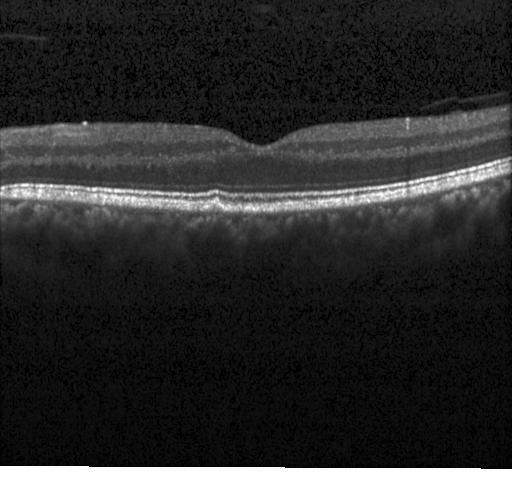 Heidelberg Spectralis OCT system. SD-OCT. Horizontal scan through the fovea. Retinal OCT cross-section.
Sub-RPE drusenoid deposits.